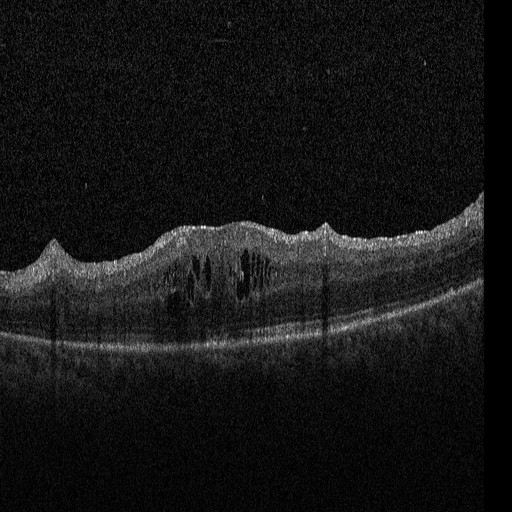 OCT line scan. SD-OCT. Acquired on a Heidelberg Spectralis. Horizontal scan through the fovea. This B-scan demonstrates diabetic macular edema (DME).